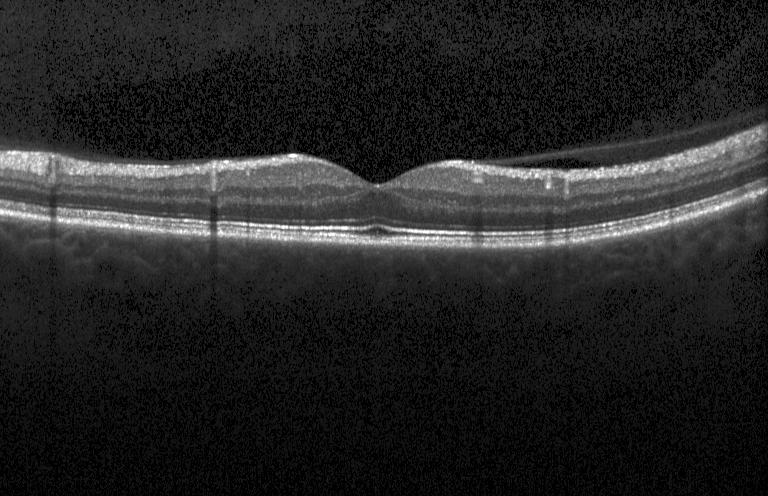

Instrument: Heidelberg Spectralis, optical coherence tomography scan, horizontal scan through the fovea, SD-OCT — OCT finding: no CNV, no DME, and no drusen.